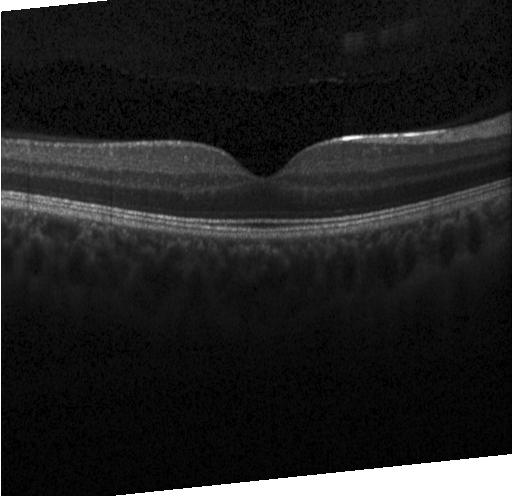

Spectral-domain OCT B-scan: neither choroidal neovascularization, diabetic macular edema, nor drusen.